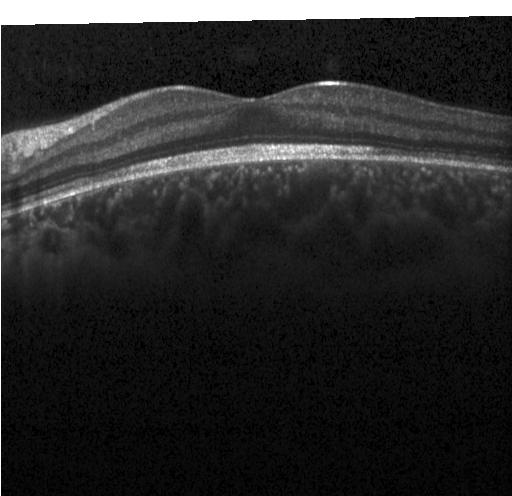

OCT B-scan · centered on the fovea · Heidelberg Spectralis OCT system · SD-OCT
Assessment: no CNV, DME, or drusen.